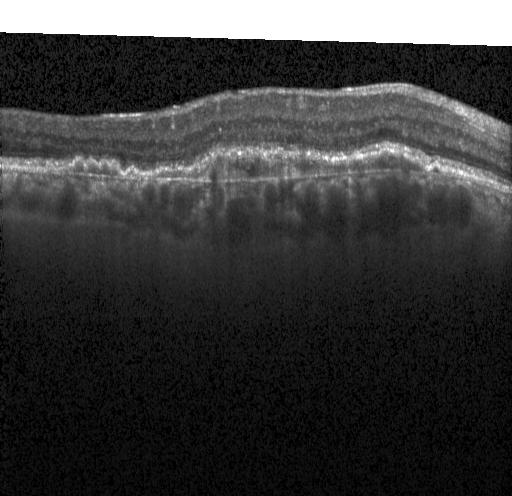
Spectral-domain OCT, OCT line scan, acquired on a Heidelberg Spectralis.
This B-scan demonstrates CNV.